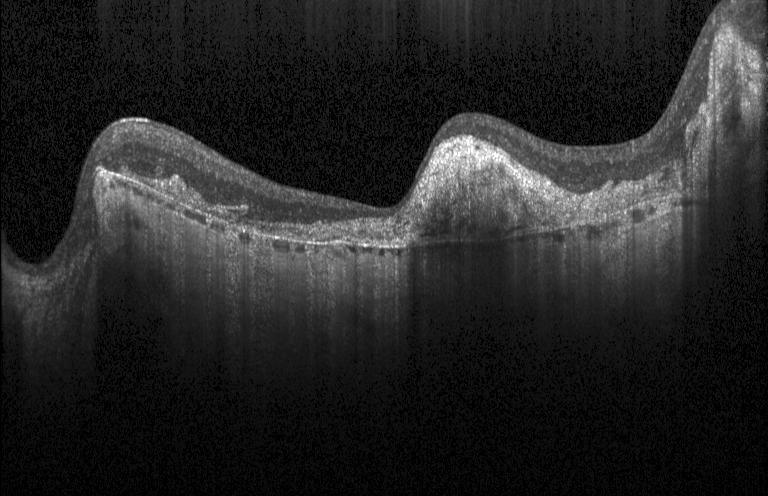 OCT B-scan showing a choroidal neovascular membrane.